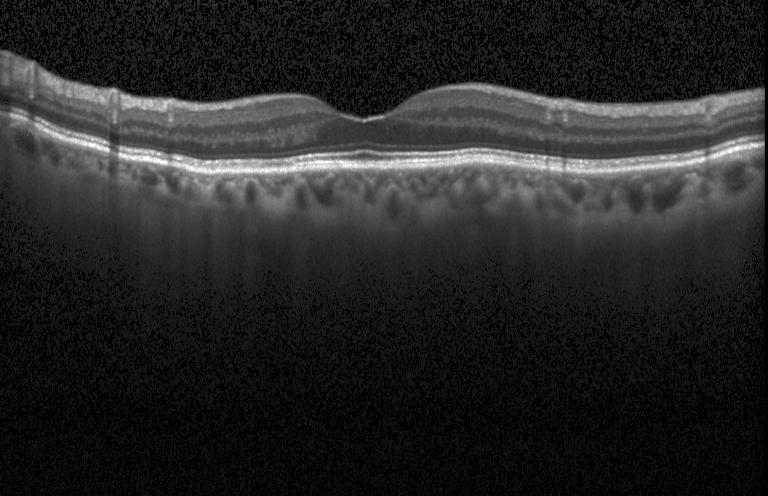 OCT finding: no choroidal neovascularization, diabetic macular edema, or drusen.